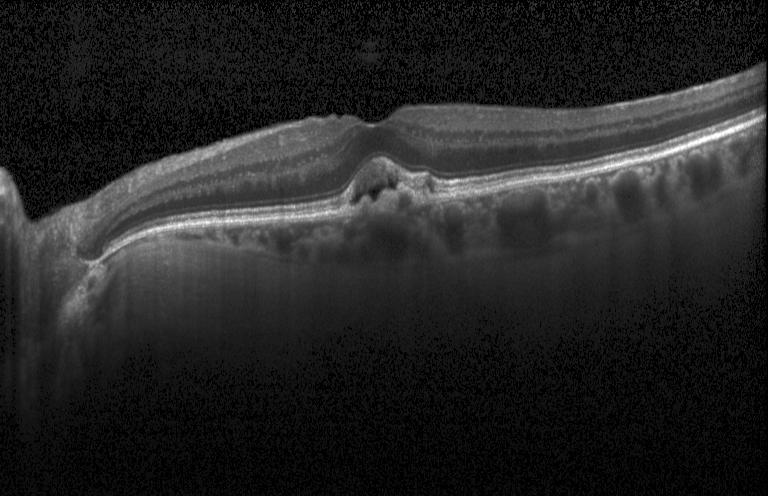 Macular OCT demonstrating choroidal neovascularization (CNV).